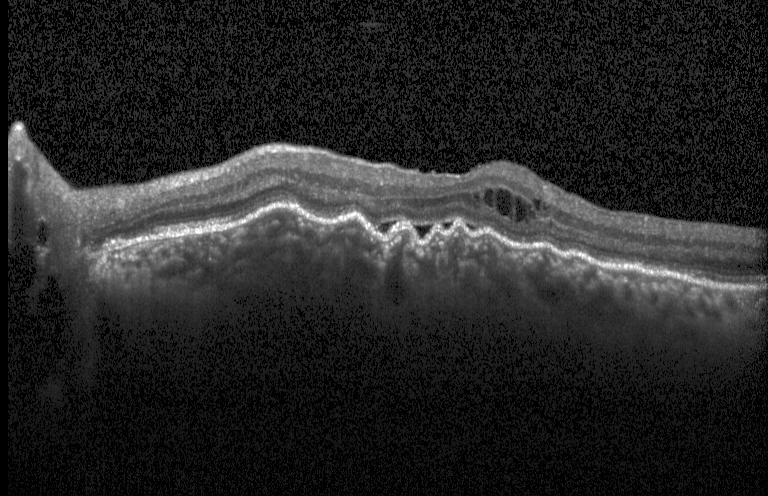
Acquired on a Heidelberg Spectralis · SD-OCT · optical coherence tomography B-scan — The scan shows a choroidal neovascular membrane.